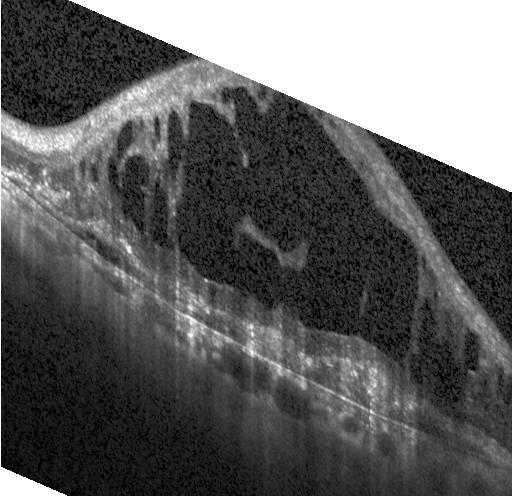 Macular OCT: CNV.